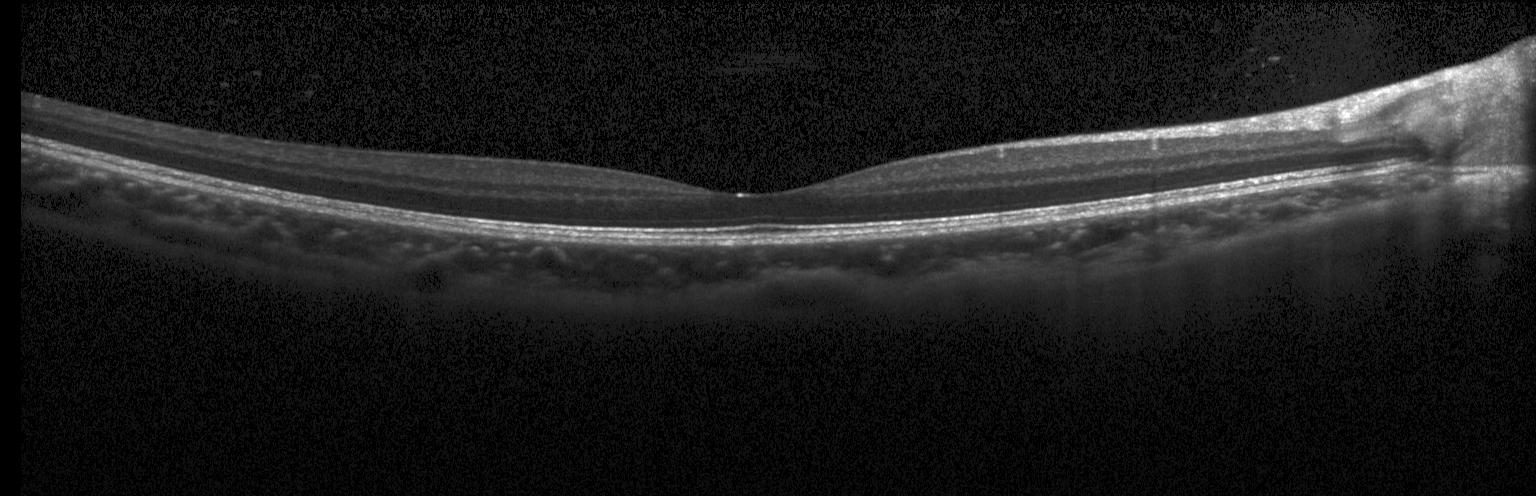

Optical coherence tomography scan. Diagnosis: no choroidal neovascularization, no diabetic macular edema, and no drusen.